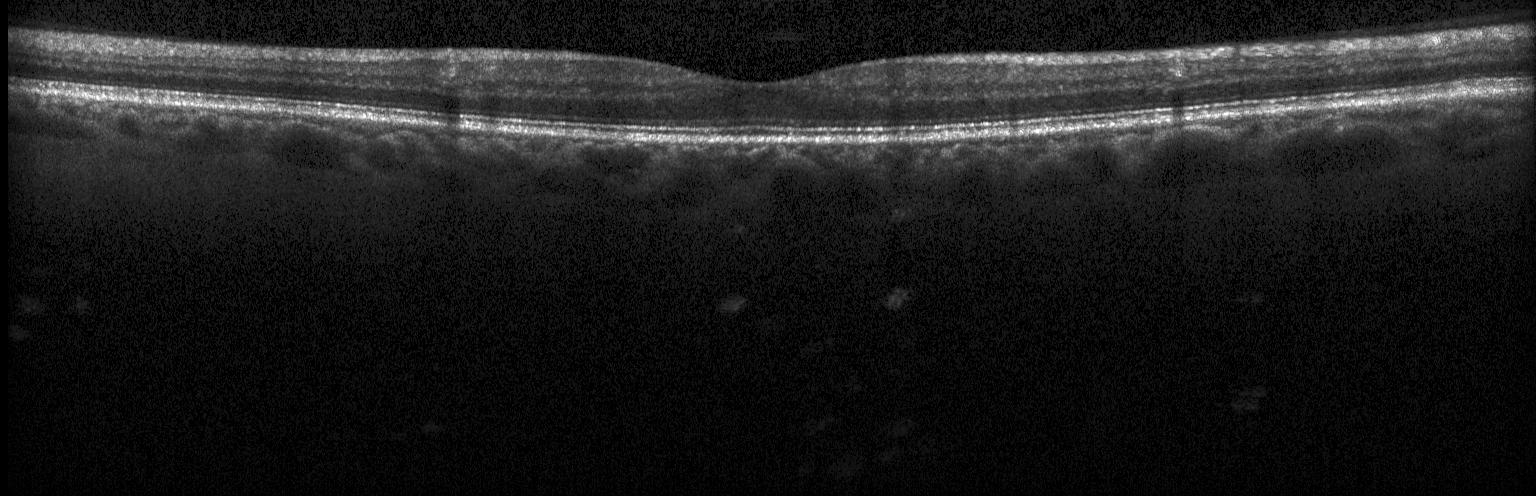
Spectral-domain OCT · centered on the fovea · OCT line scan. Diagnosis: no choroidal neovascularization, diabetic macular edema, or drusen.